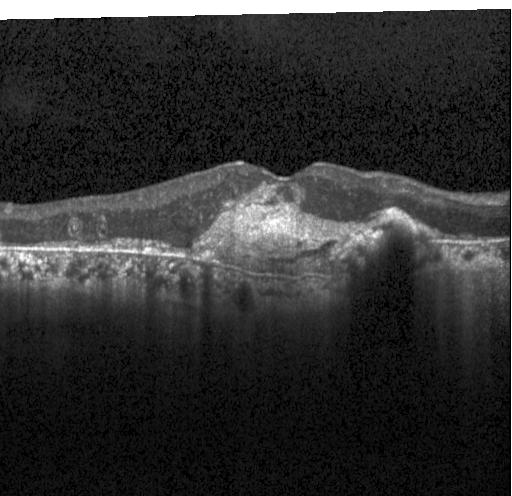 Spectral-domain optical coherence tomography, retinal OCT B-scan, acquired on a Heidelberg Spectralis. Assessment: choroidal neovascularization (CNV).